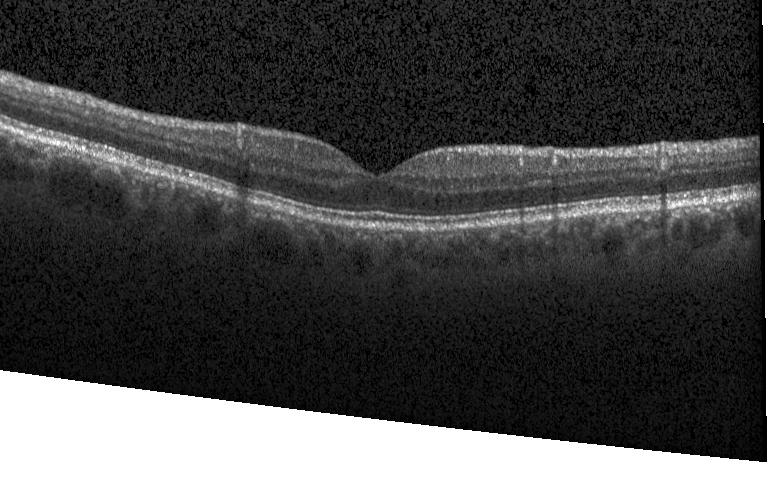
Impression: neither choroidal neovascularization, diabetic macular edema, nor drusen.